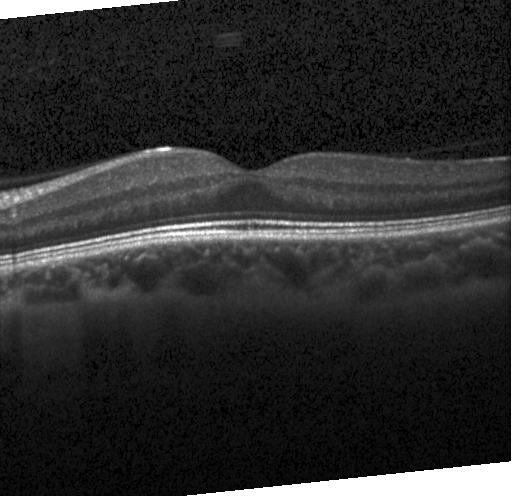 Optical coherence tomography scan
Diagnosis: neither choroidal neovascularization, diabetic macular edema, nor drusen.